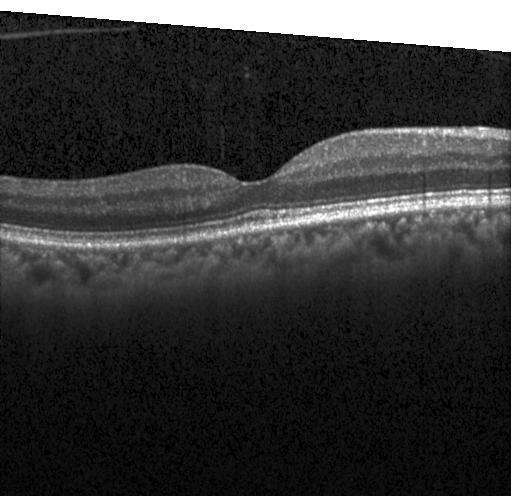
Dx: no CNV, no DME, and no drusen.